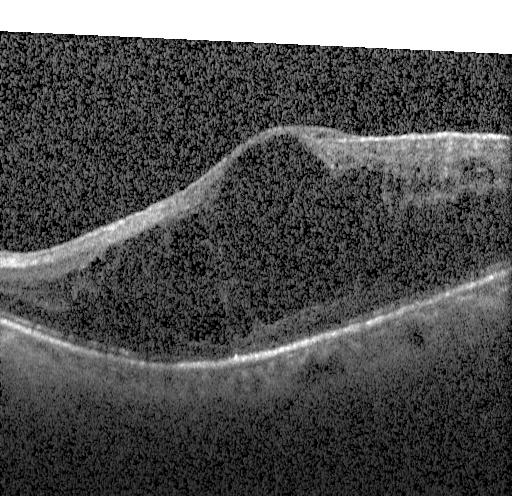
Through the macula · optical coherence tomography scan.
Assessment: diabetic macular edema.